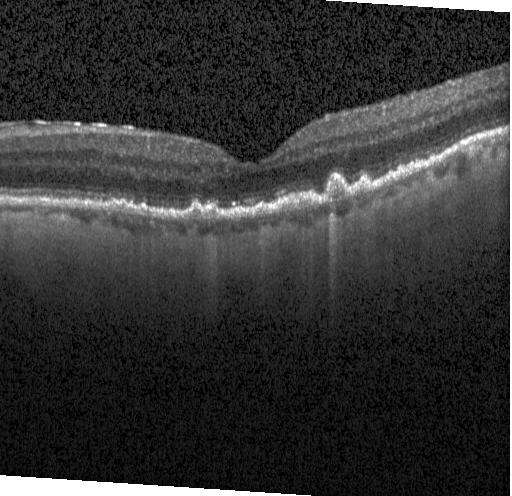
OCT B-scan; acquired on a Heidelberg Spectralis.
Assessment: drusen.